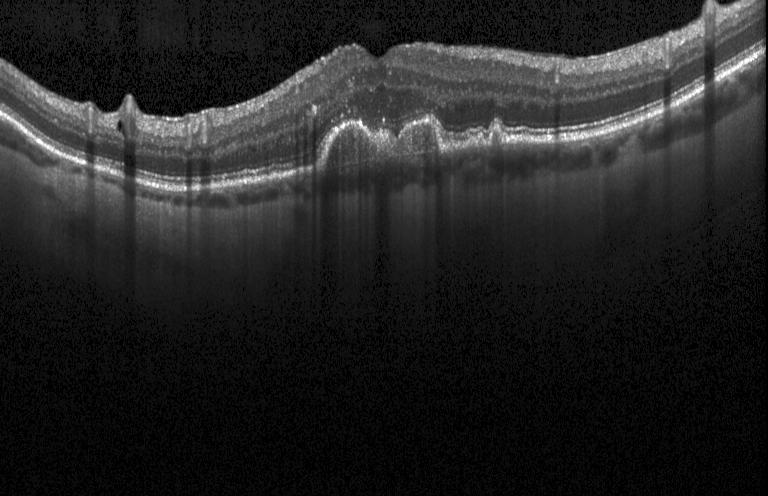 Finding: multiple drusen.